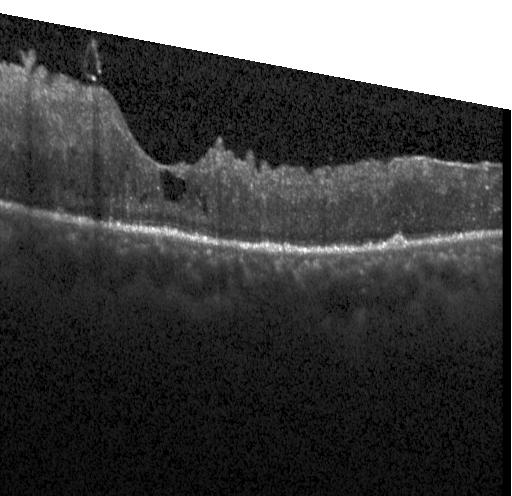 Spectral-domain optical coherence tomography, optical coherence tomography B-scan
Impression: diabetic macular edema (DME).